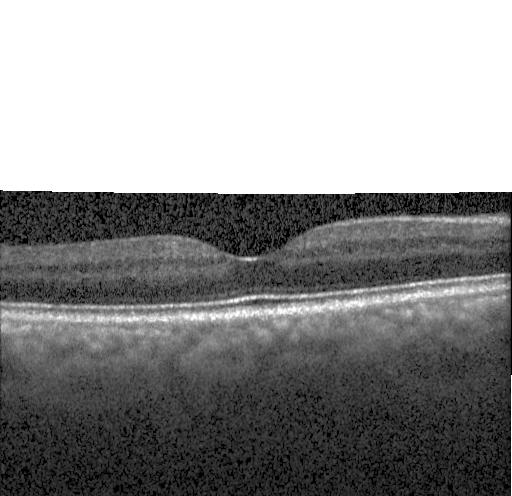
Dx: neither choroidal neovascularization, diabetic macular edema, nor drusen.